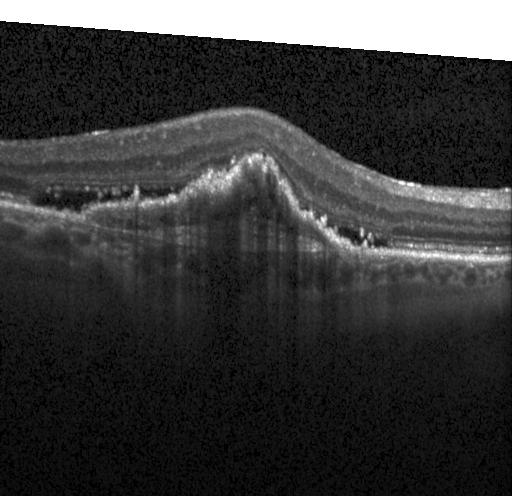
Diagnosis: a choroidal neovascular membrane.